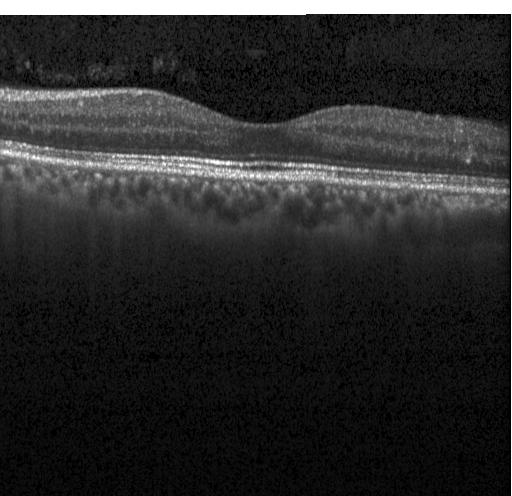 Heidelberg Spectralis; OCT B-scan; centered on the fovea — The scan shows no choroidal neovascularization, no diabetic macular edema, and no drusen.